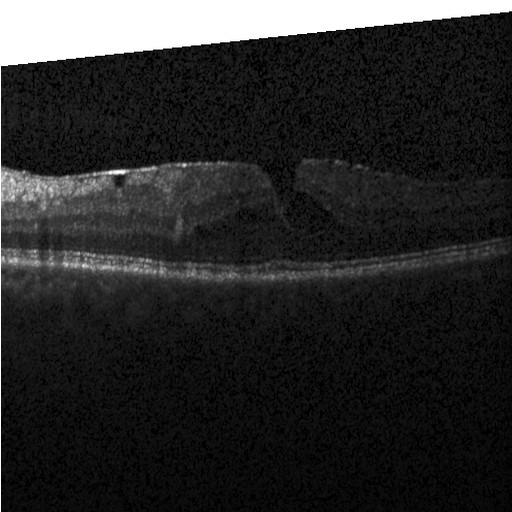
Macular OCT: DME.